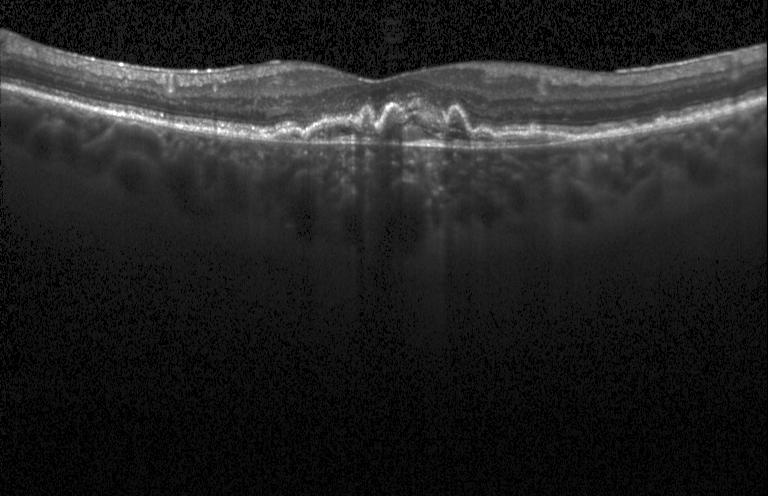 Retinal OCT B-scan. Through the macula. Heidelberg Spectralis.
Macular OCT: a choroidal neovascular membrane.